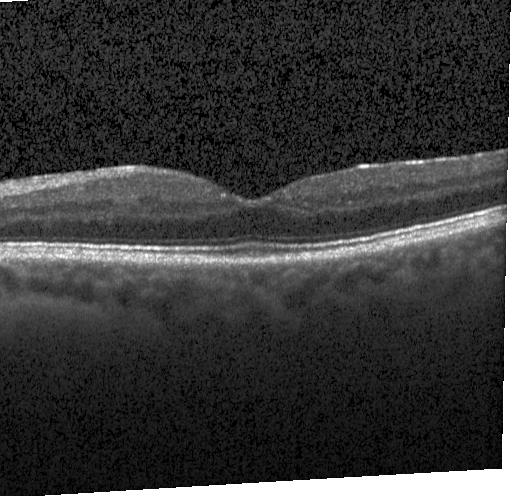

Optical coherence tomography B-scan.
Finding: neither choroidal neovascularization, diabetic macular edema, nor drusen.